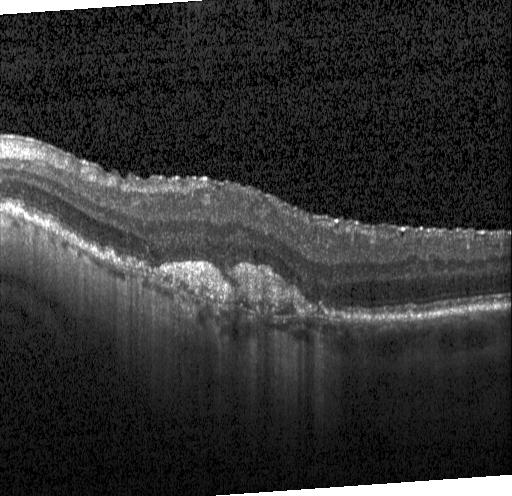 Retinal OCT B-scan.
Diagnosis: a choroidal neovascular membrane.